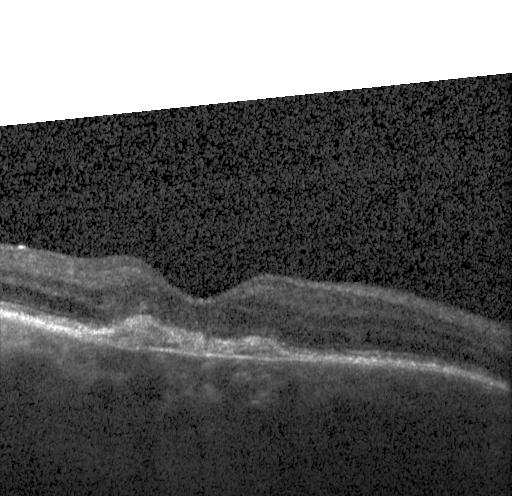

Finding: CNV.